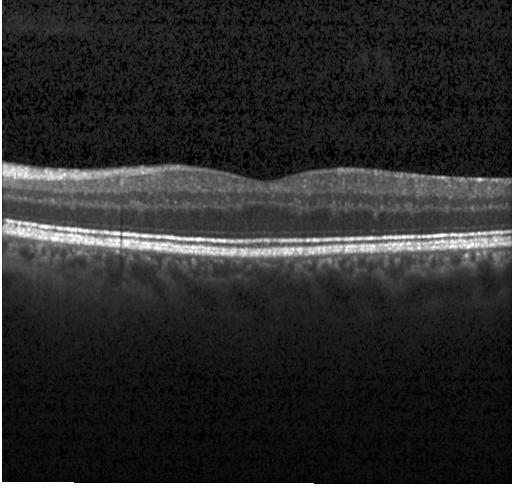 Instrument: Heidelberg Spectralis. Spectral-domain optical coherence tomography. Retinal OCT B-scan
This B-scan demonstrates no choroidal neovascularization, diabetic macular edema, or drusen.